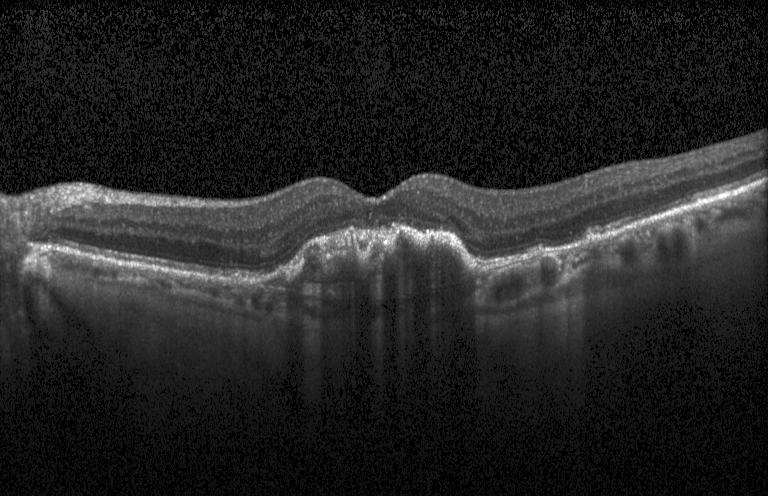

Acquired on a Heidelberg Spectralis; macular scan; OCT line scan
Macular OCT: a choroidal neovascular membrane.